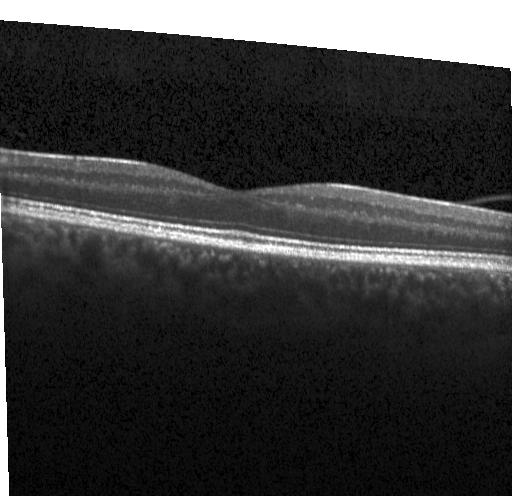
Spectral-domain OCT, optical coherence tomography scan, instrument: Heidelberg Spectralis
This B-scan demonstrates no choroidal neovascularization, diabetic macular edema, or drusen.